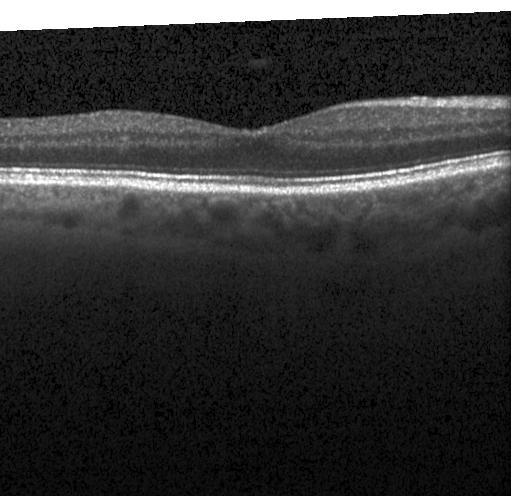 Optical coherence tomography scan; Heidelberg Spectralis OCT system; macular scan
Impression: neither CNV, DME, nor drusen.